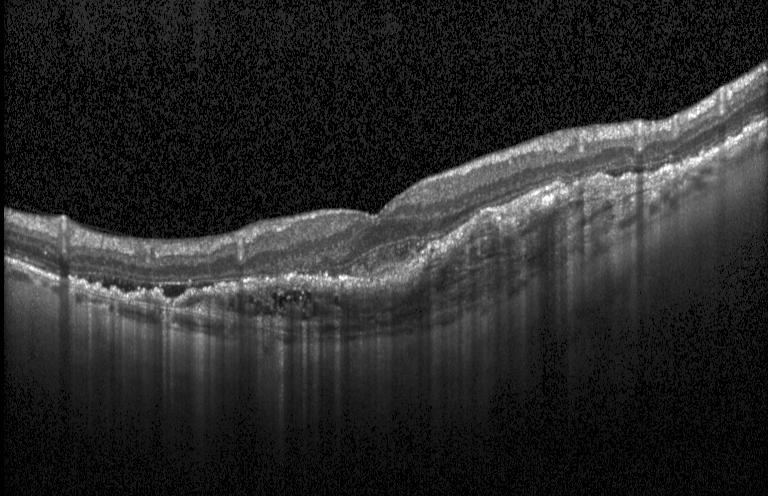 Optical coherence tomography B-scan; through the macula
Finding: a choroidal neovascular membrane.